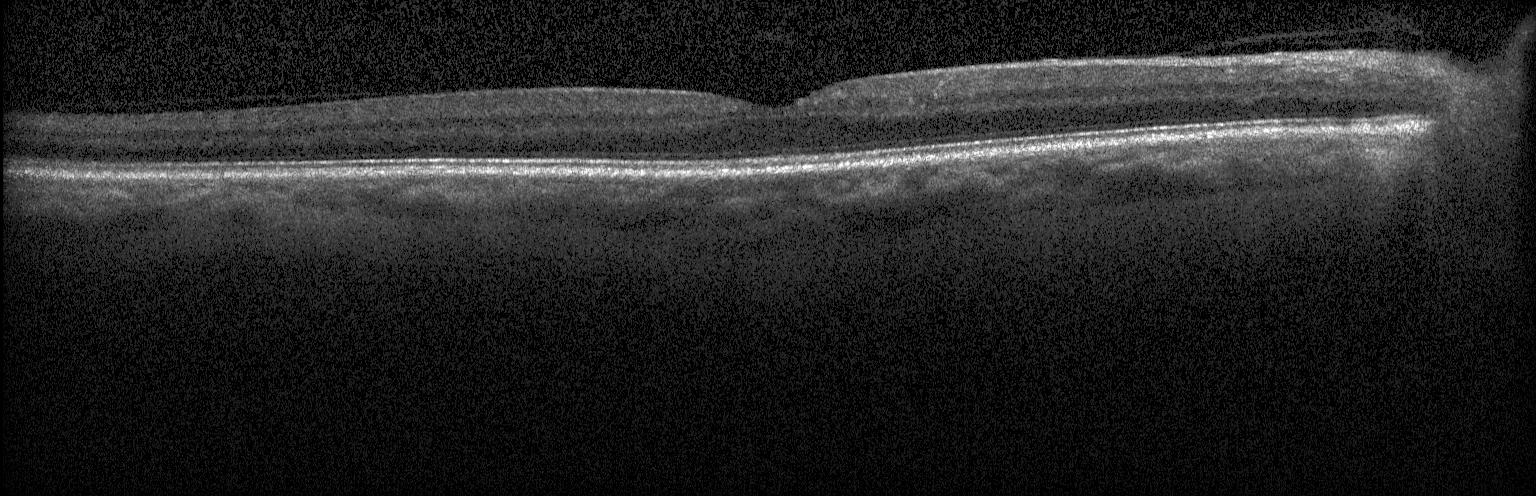
Optical coherence tomography B-scan — The scan shows neither CNV, DME, nor drusen.